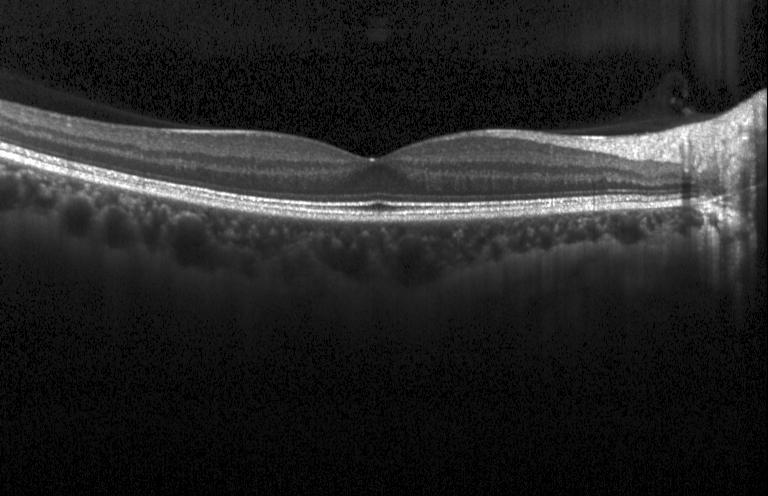 Retinal OCT B-scan
Diagnosis: no CNV, no DME, and no drusen.